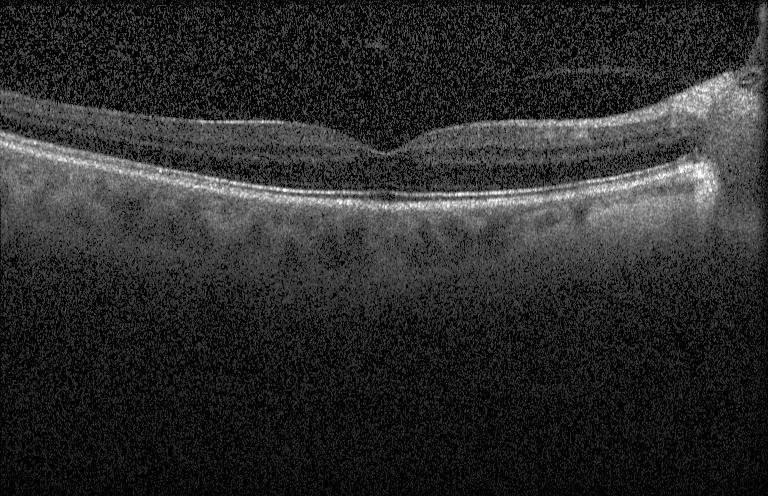 Instrument: Heidelberg Spectralis; retinal OCT B-scan
Impression: no choroidal neovascularization, diabetic macular edema, or drusen.